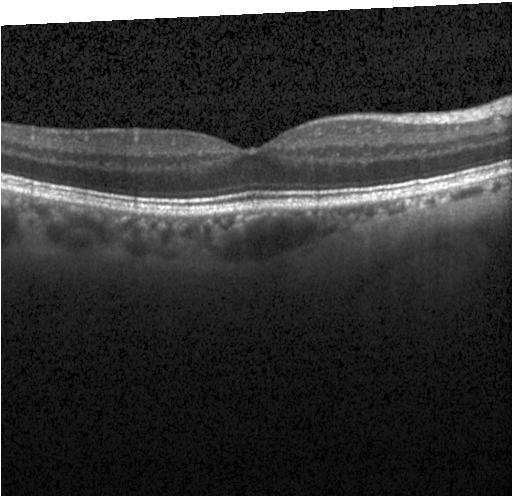 OCT scan showing no choroidal neovascularization, no diabetic macular edema, and no drusen.